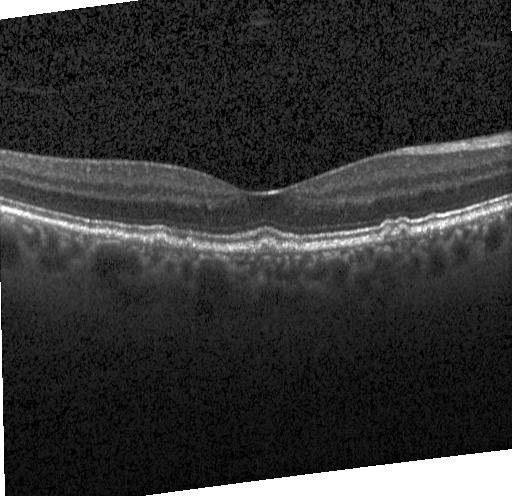

Impression: multiple drusen.